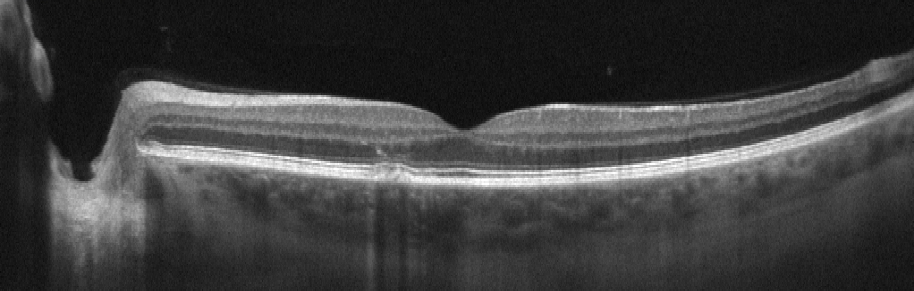 OCT B-scan · OS. Finding: age-related macular degeneration (AMD).